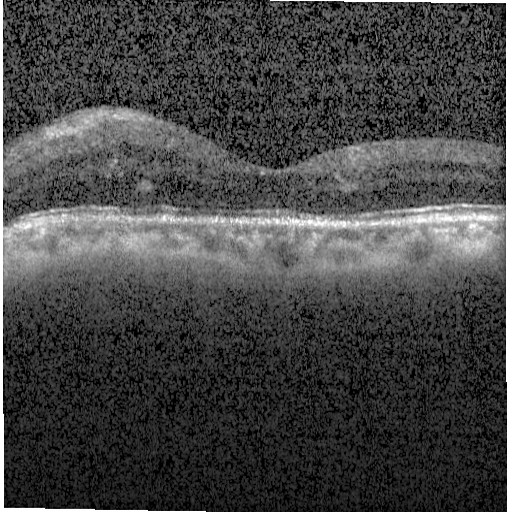

Centered on the fovea, retinal OCT cross-section, spectral-domain OCT
Impression: diabetic macular edema.